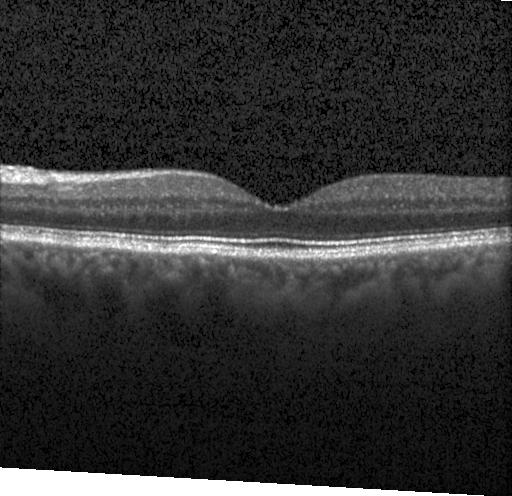

Retinal OCT cross-section showing no choroidal neovascularization, no diabetic macular edema, and no drusen.